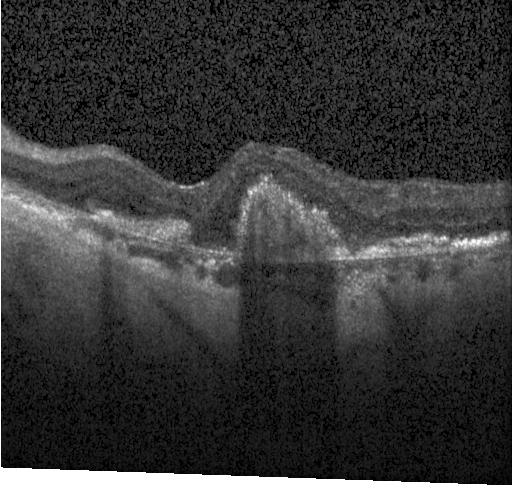 Optical coherence tomography scan · fovea-centered · SD-OCT · acquired on a Heidelberg Spectralis
Finding: CNV.